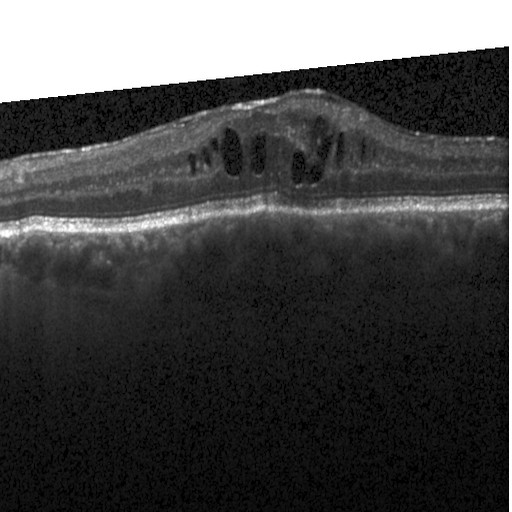

OCT finding: diabetic macular edema (DME).